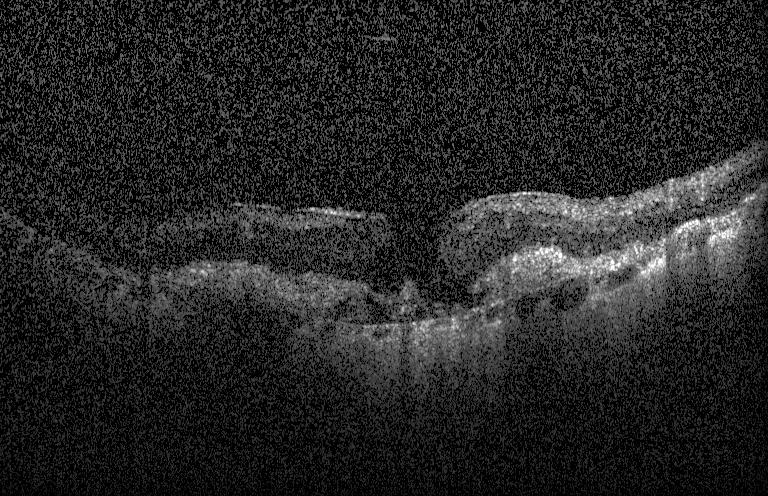
Dx: CNV.